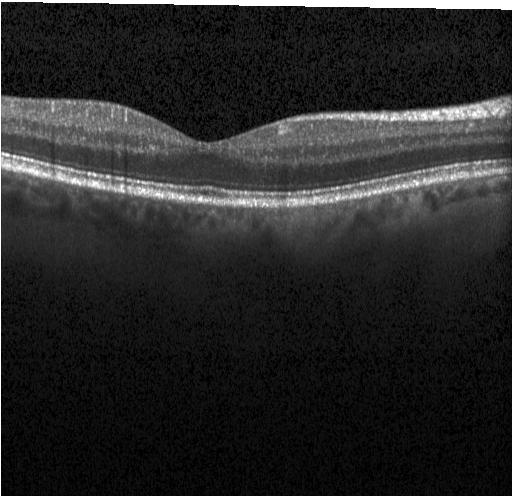 Heidelberg Spectralis OCT system; SD-OCT; OCT B-scan. The scan shows neither choroidal neovascularization, diabetic macular edema, nor drusen.